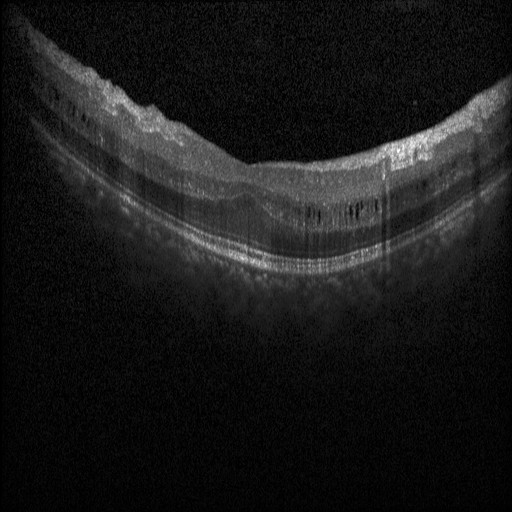 Spectral-domain optical coherence tomography; macular scan; retinal OCT B-scan. This B-scan demonstrates DME.